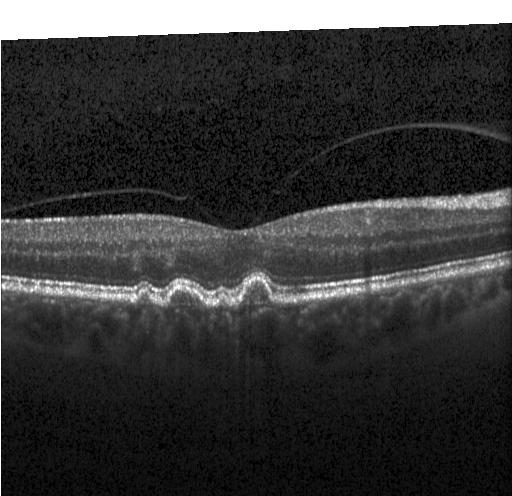 OCT scan showing drusen.